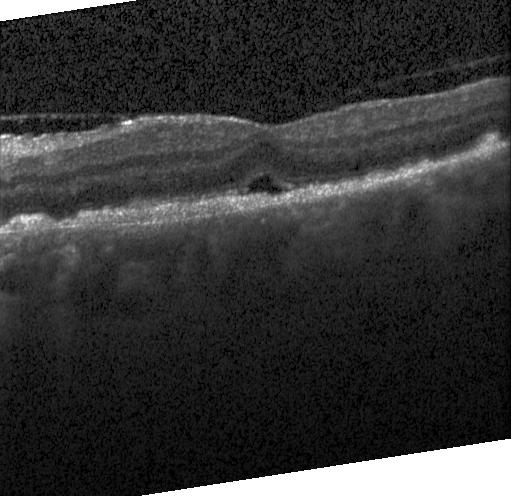 Centered on the fovea, retinal OCT B-scan — Diagnosis: CNV.